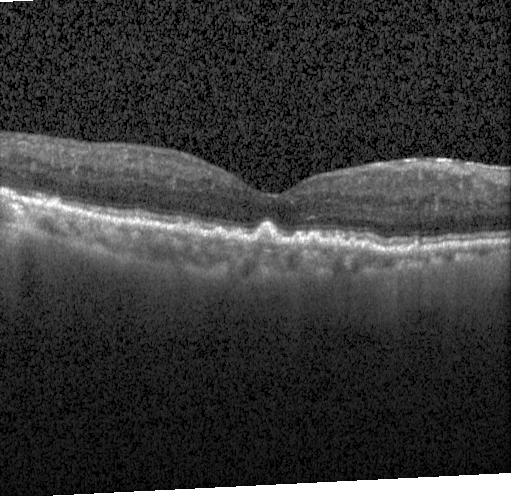 OCT line scan · through the macula · Heidelberg Spectralis · spectral-domain optical coherence tomography — Finding: sub-RPE drusenoid deposits.